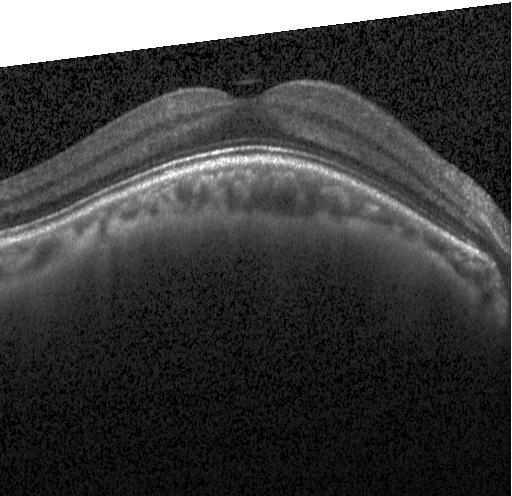

Diagnosis: no evidence of choroidal neovascularization, diabetic macular edema, or drusen.